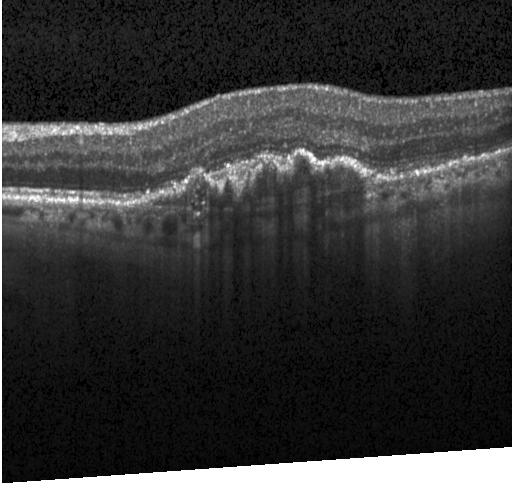
Diagnosis: choroidal neovascularization (CNV).